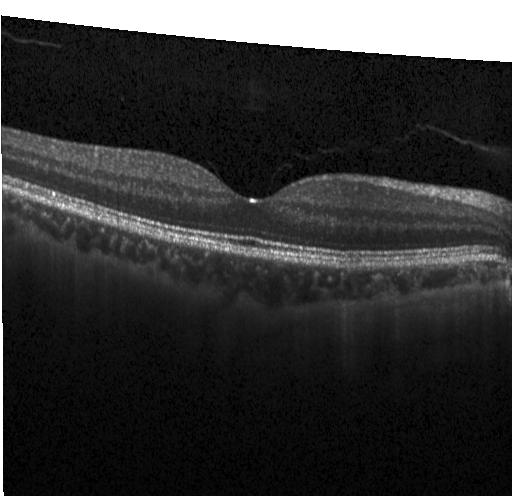
Spectral-domain OCT B-scan: no evidence of choroidal neovascularization, diabetic macular edema, or drusen.